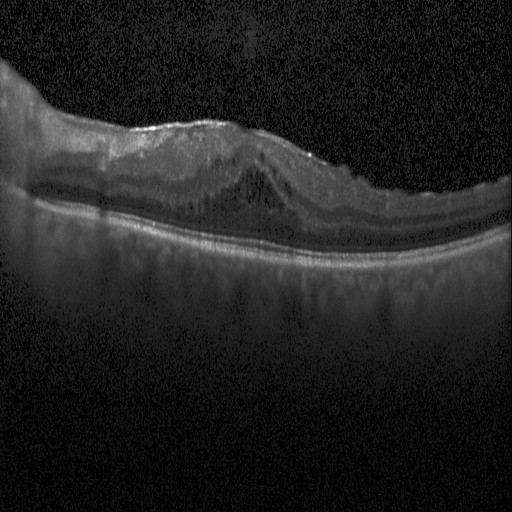

Heidelberg Spectralis OCT system. Retinal OCT B-scan — Dx: DME.